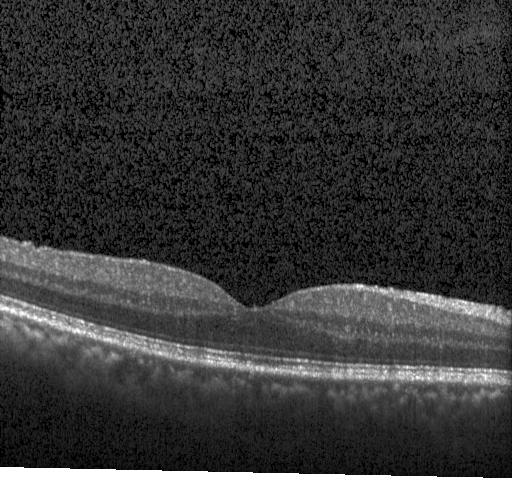 Horizontal scan through the fovea. Spectral-domain optical coherence tomography. OCT B-scan. Heidelberg Spectralis
The scan shows no CNV, no DME, and no drusen.